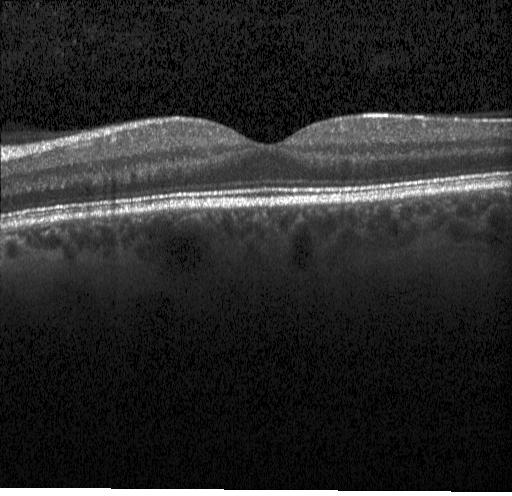
Centered on the fovea. OCT line scan
Impression: no CNV, no DME, and no drusen.